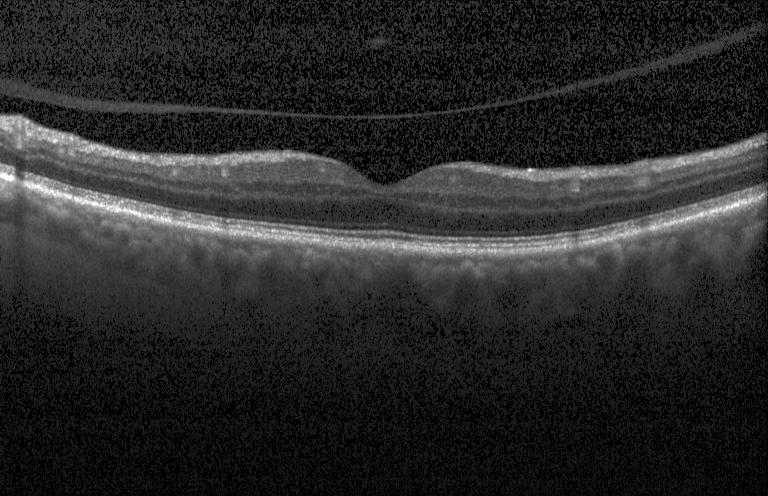 Macular OCT: neither choroidal neovascularization, diabetic macular edema, nor drusen.